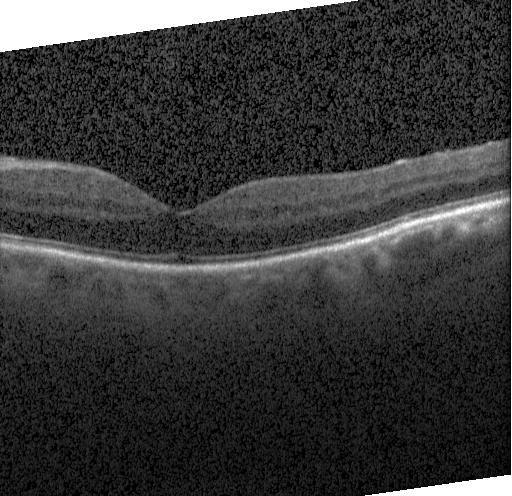 Finding: neither CNV, DME, nor drusen.